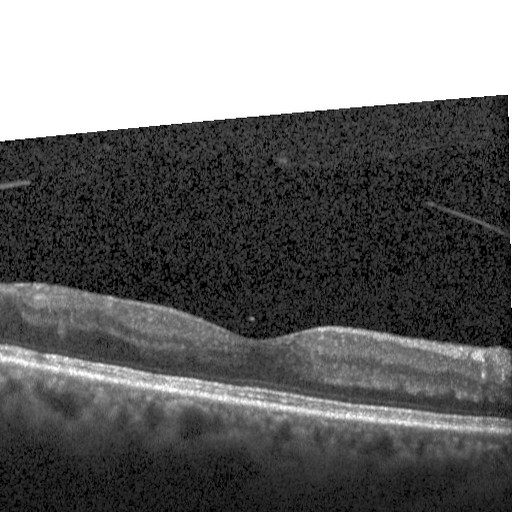 Macular OCT demonstrating diabetic macular edema.